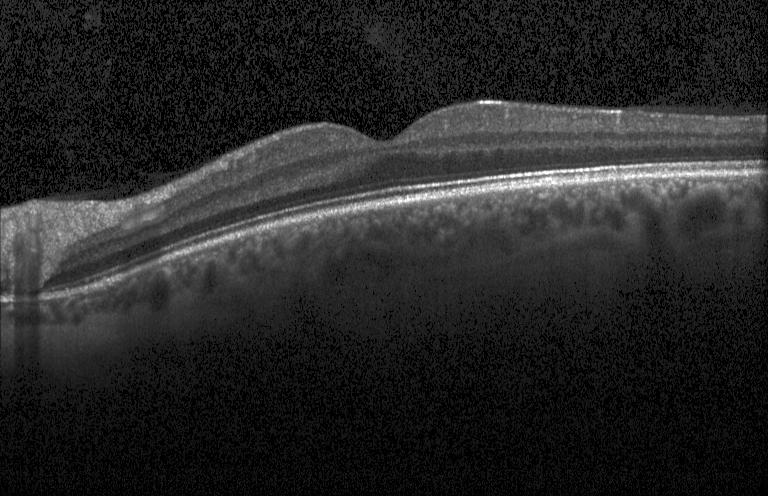

SD-OCT. Heidelberg Spectralis. Optical coherence tomography scan. Macular scan — Assessment: no choroidal neovascularization, diabetic macular edema, or drusen.